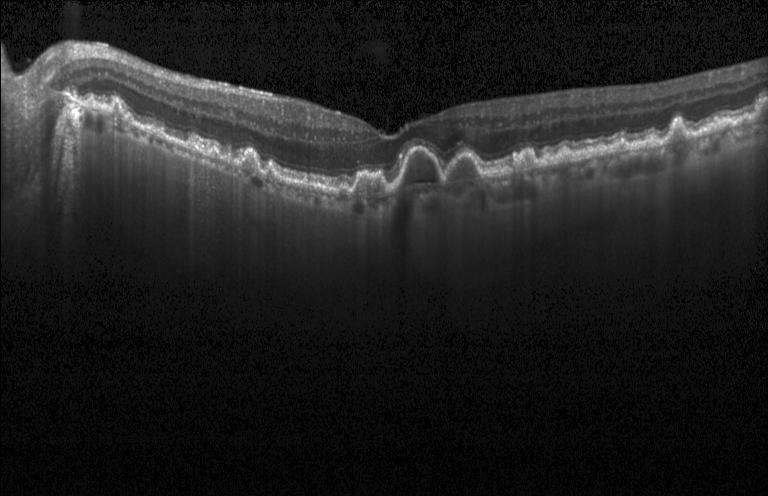

Retinal OCT B-scan; spectral-domain optical coherence tomography; through the macula; Heidelberg Spectralis OCT system. OCT finding: sub-RPE drusenoid deposits.